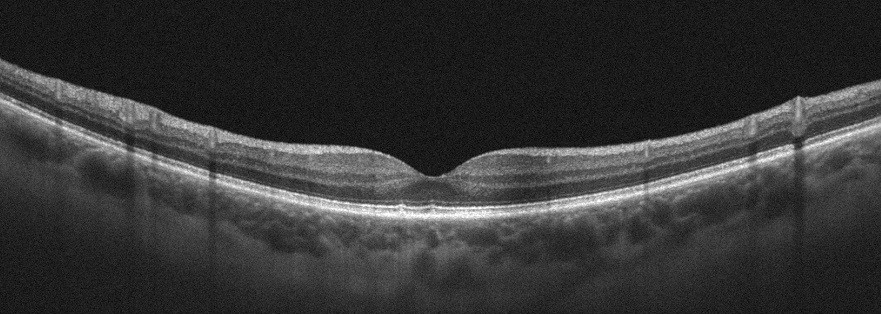

OCT line scan.
Impression: age-related macular degeneration (AMD).